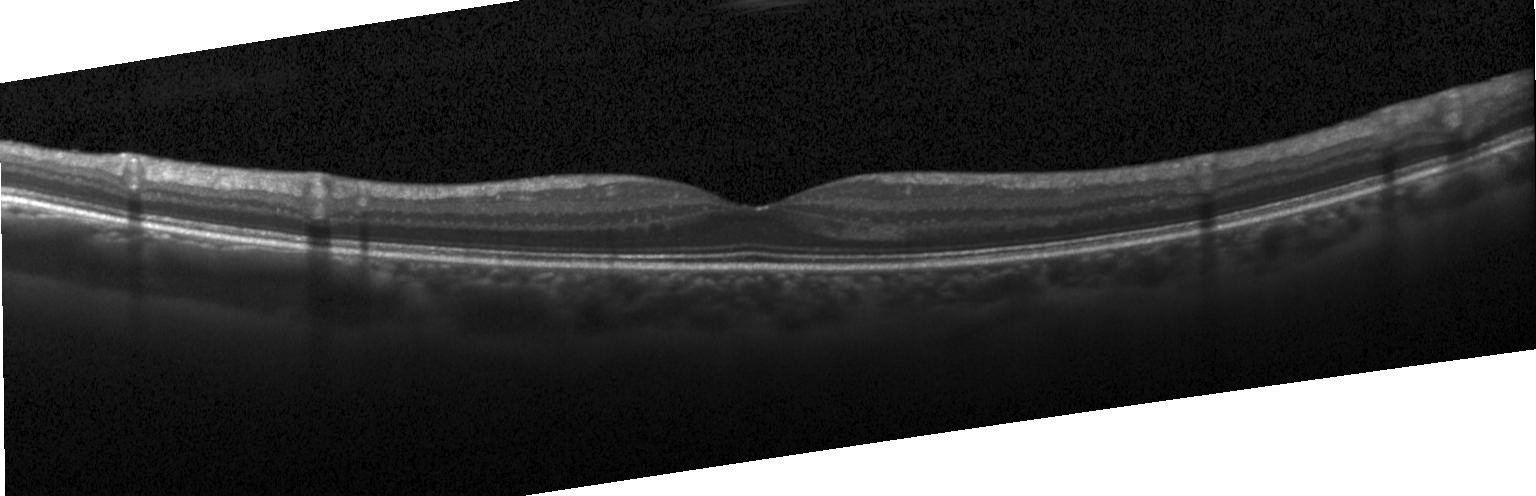
Spectral-domain optical coherence tomography · OCT B-scan · centered on the fovea.
Impression: no choroidal neovascularization, no diabetic macular edema, and no drusen.